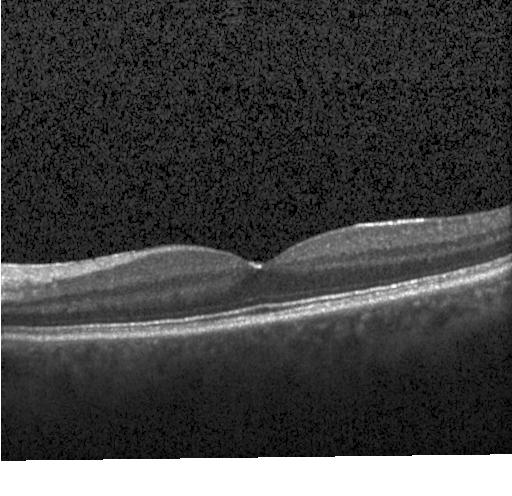
SD-OCT · retinal OCT B-scan · instrument: Heidelberg Spectralis
Macular OCT: no choroidal neovascularization, diabetic macular edema, or drusen.